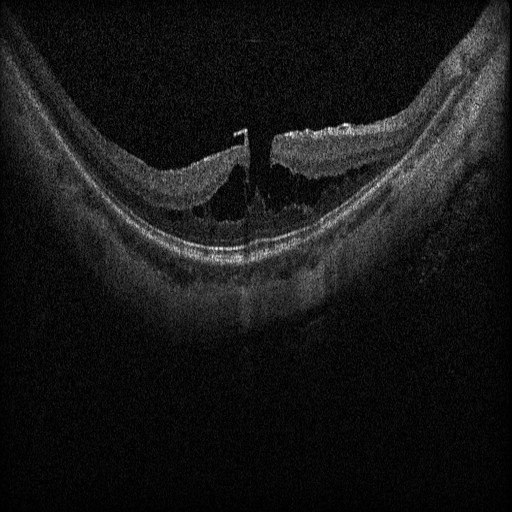
Retinal OCT cross-section. Diagnosis: DME.